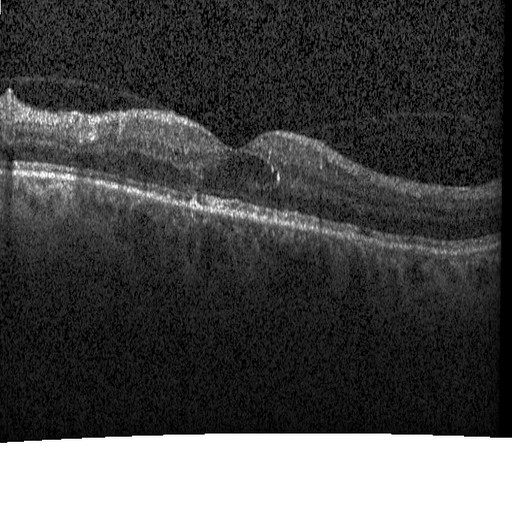
OCT finding: DME.